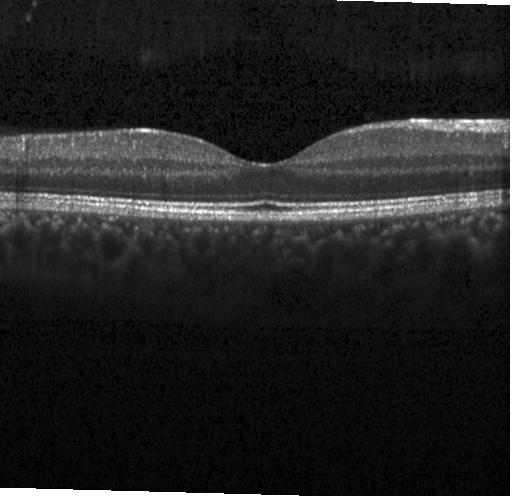 Optical coherence tomography B-scan, centered on the fovea, Heidelberg Spectralis OCT system, spectral-domain optical coherence tomography
OCT finding: no choroidal neovascularization, no diabetic macular edema, and no drusen.